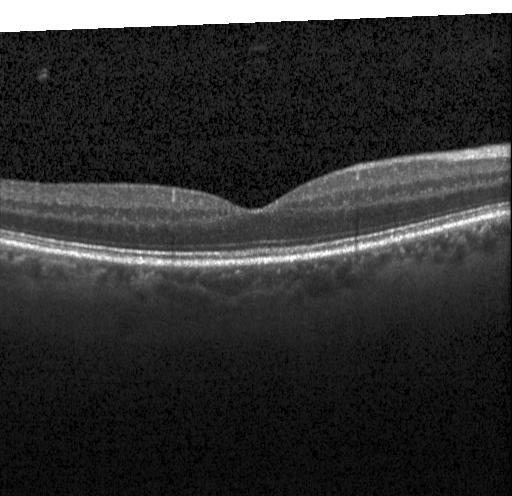
Macular OCT demonstrating no CNV, no DME, and no drusen.